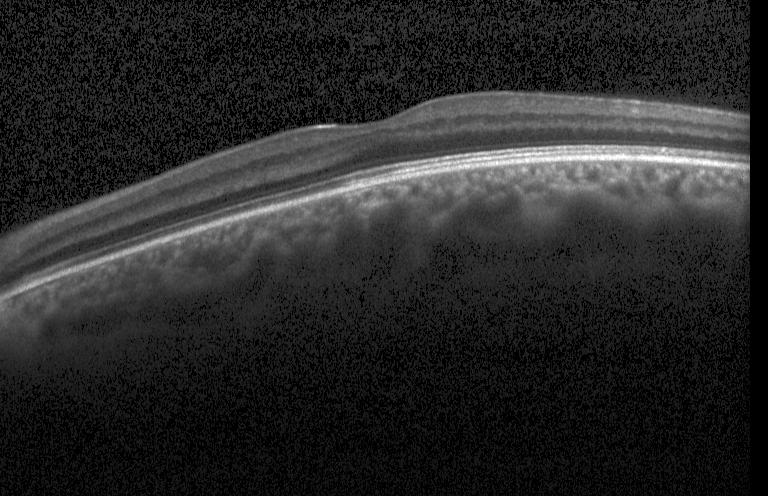
Spectral-domain OCT. Through the macula. OCT line scan
Diagnosis: no CNV, no DME, and no drusen.